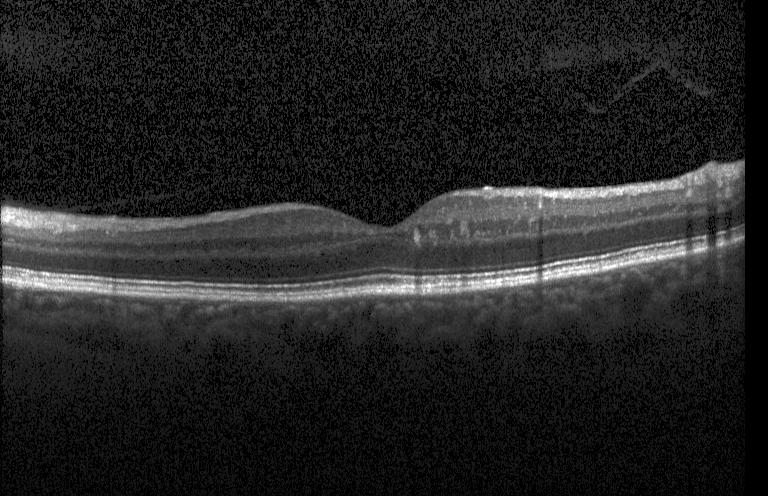 Centered on the fovea; optical coherence tomography scan; Heidelberg Spectralis; spectral-domain OCT.
The scan shows no choroidal neovascularization, diabetic macular edema, or drusen.